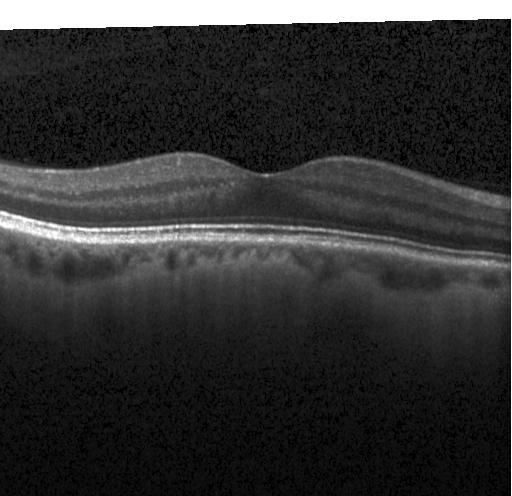

Retinal OCT cross-section showing neither choroidal neovascularization, diabetic macular edema, nor drusen.